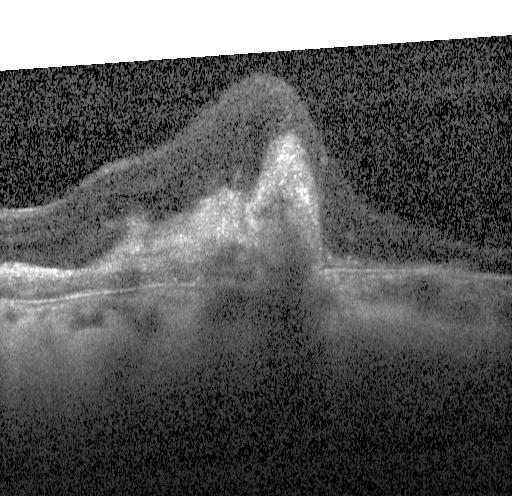
Optical coherence tomography B-scan.
Diagnosis: a choroidal neovascular membrane.